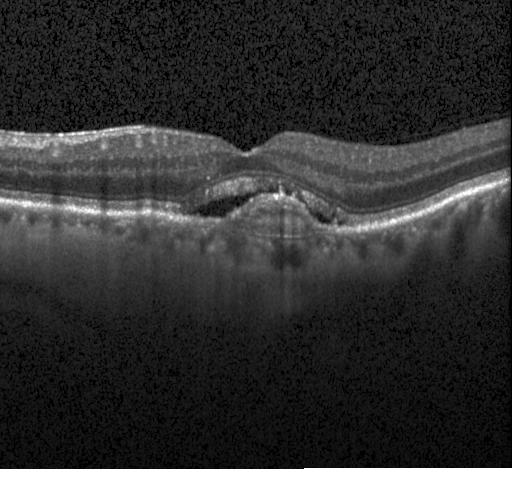
Dx: a choroidal neovascular membrane.